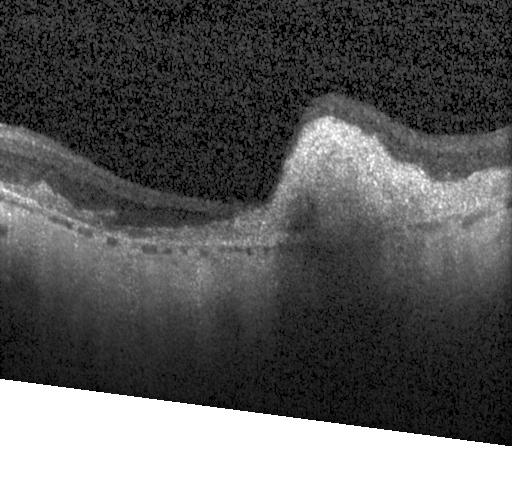 OCT finding: choroidal neovascularization (CNV).